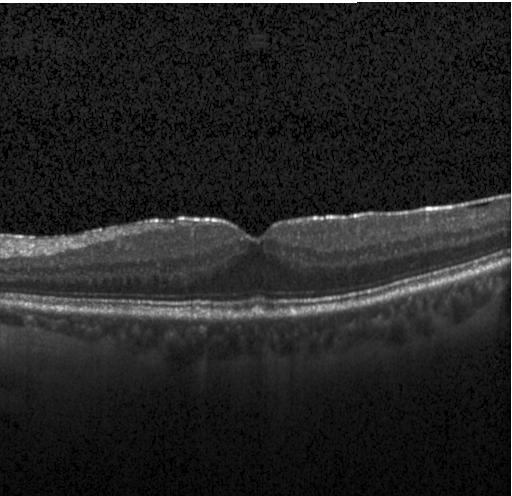
OCT finding: multiple drusen.